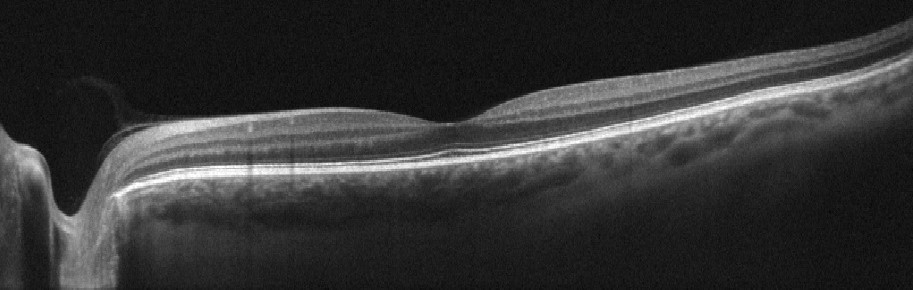
Finding: no AMD, DME, ERM, RAO, RVO, or VID.